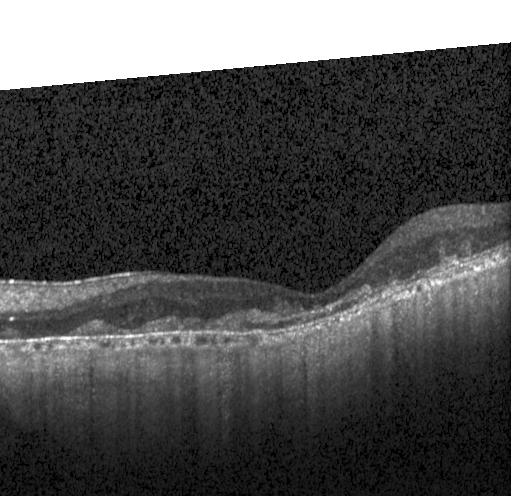
Fovea-centered; Heidelberg Spectralis OCT system; retinal OCT cross-section — Assessment: a choroidal neovascular membrane.